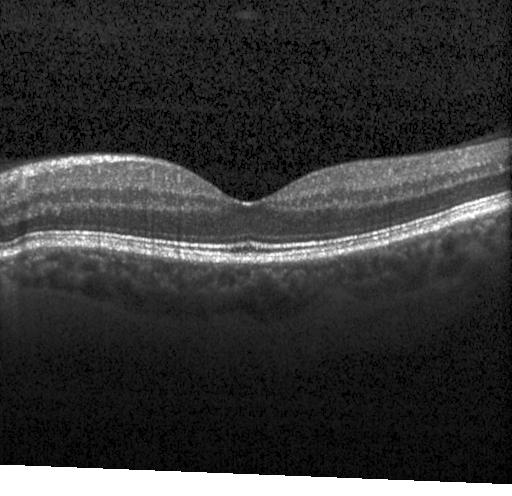
Macular OCT: no choroidal neovascularization, diabetic macular edema, or drusen.